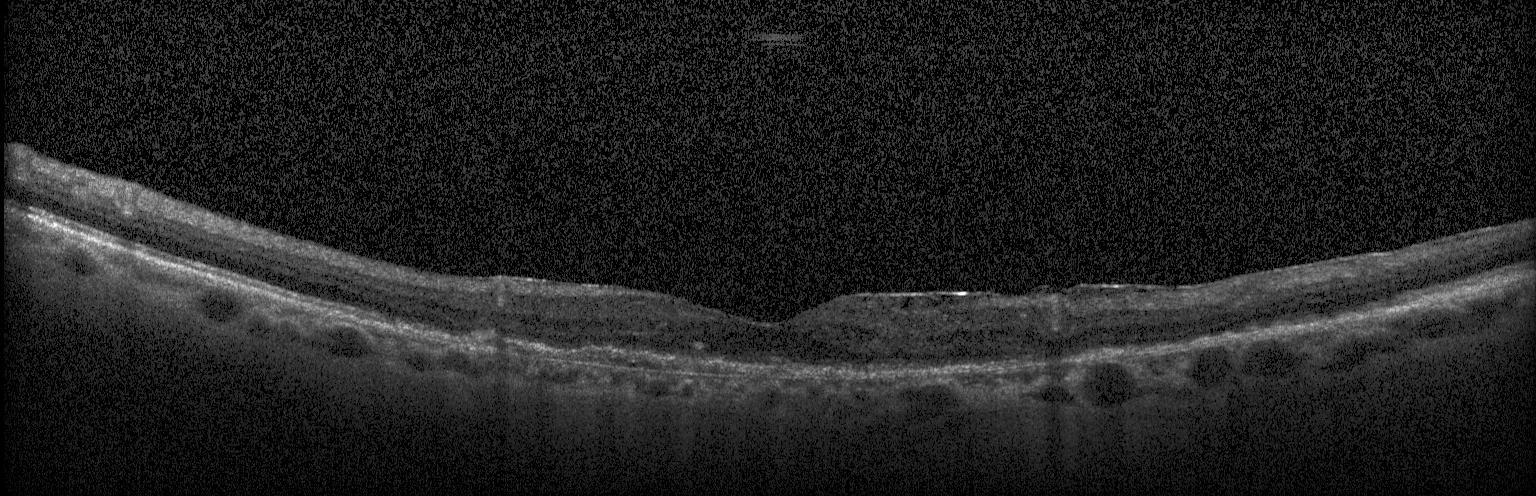
OCT line scan — Macular OCT: a choroidal neovascular membrane.